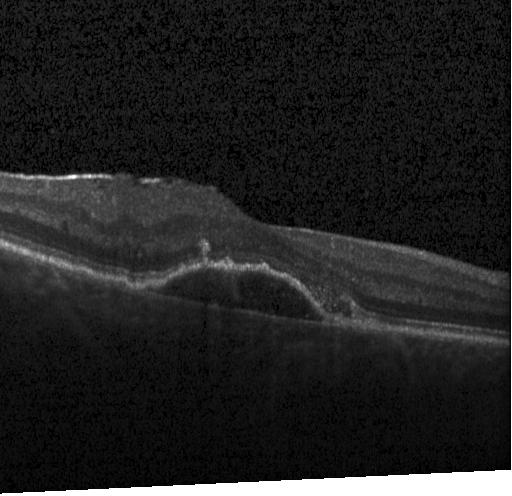
Diagnosis: choroidal neovascularization (CNV).